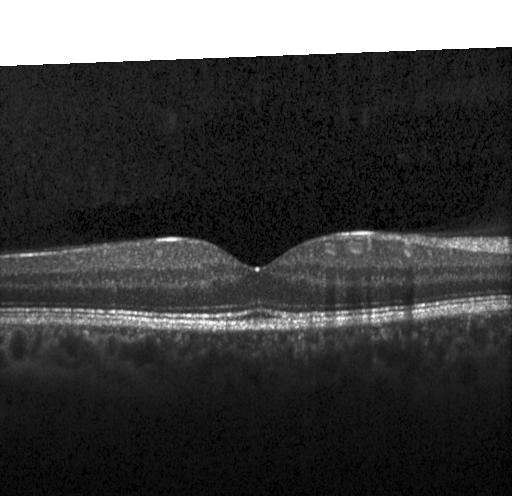
This B-scan demonstrates no evidence of choroidal neovascularization, diabetic macular edema, or drusen.